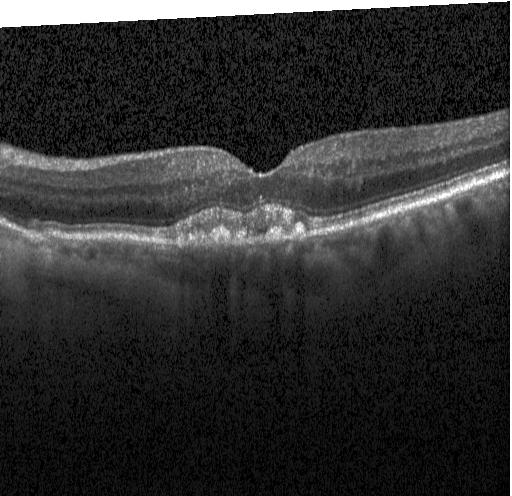
OCT finding: choroidal neovascularization.